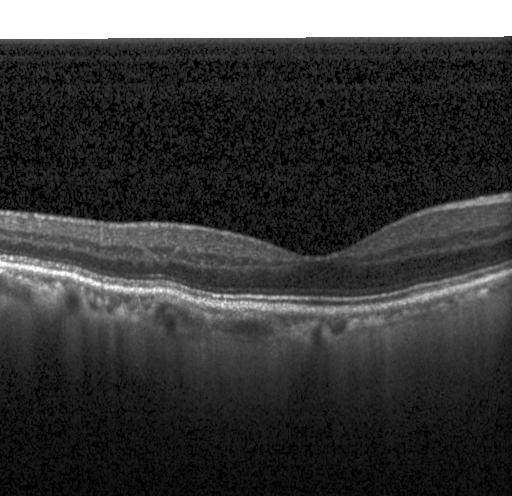
OCT B-scan.
Diagnosis: no evidence of choroidal neovascularization, diabetic macular edema, or drusen.